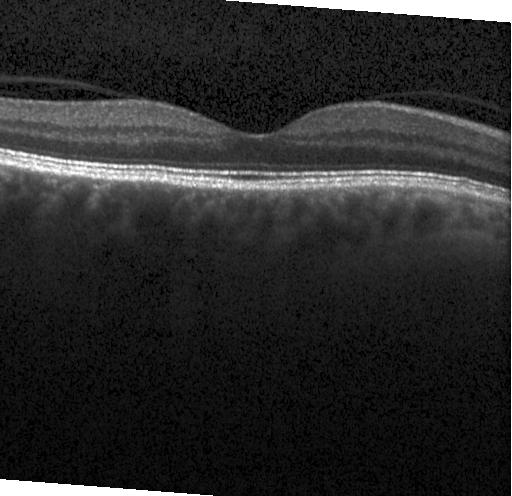
Retinal OCT B-scan. Macular scan.
Finding: neither choroidal neovascularization, diabetic macular edema, nor drusen.